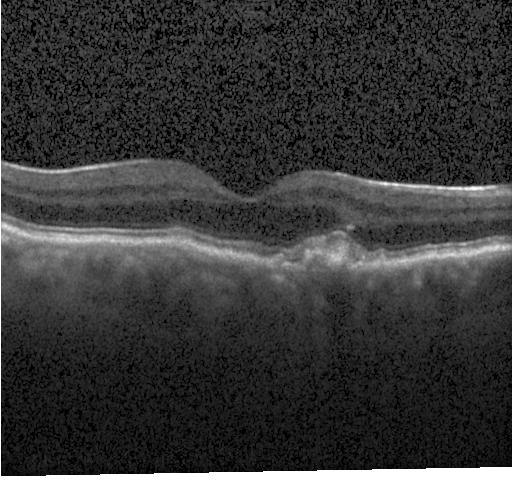

Impression: a choroidal neovascular membrane.